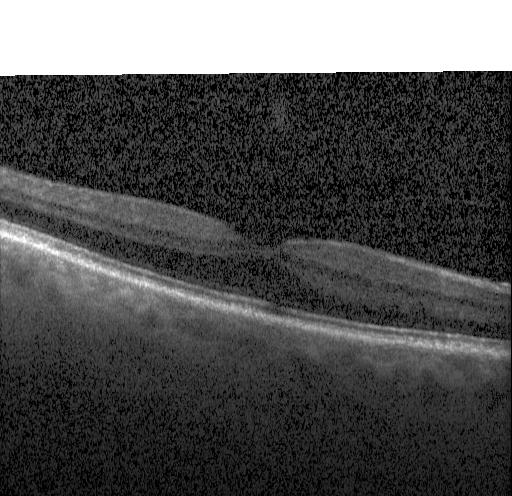

Instrument: Heidelberg Spectralis; retinal OCT cross-section. Diagnosis: neither choroidal neovascularization, diabetic macular edema, nor drusen.